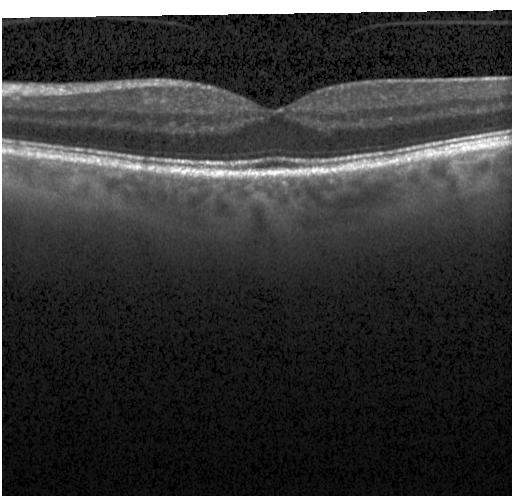
Retinal OCT cross-section showing no choroidal neovascularization, diabetic macular edema, or drusen.